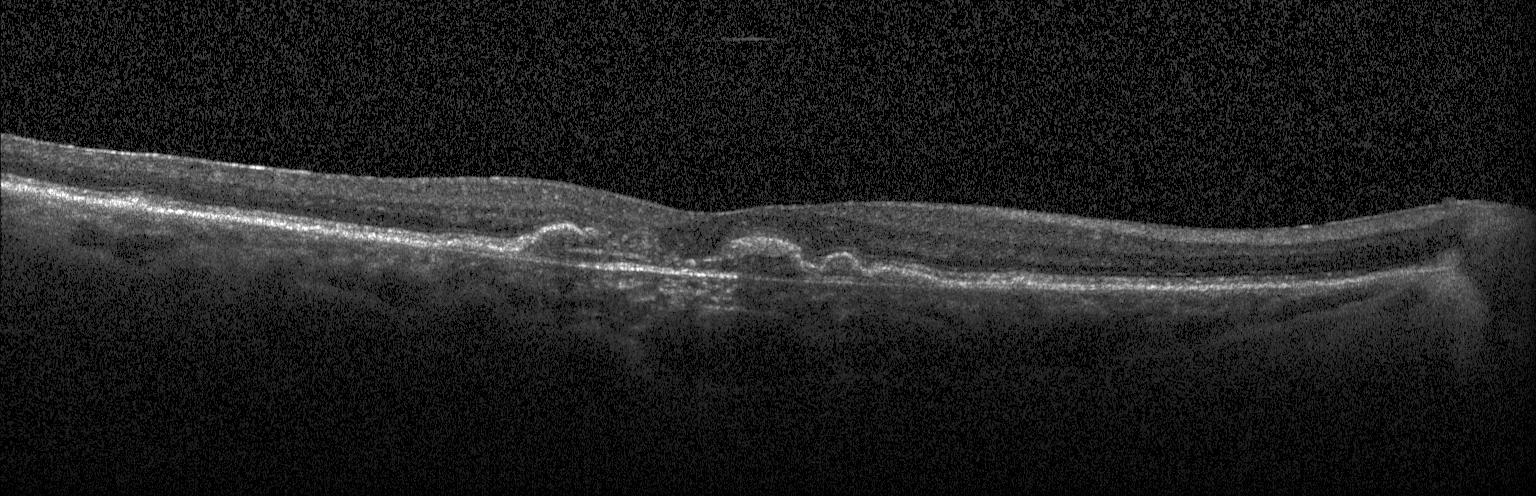 Retinal OCT cross-section, macular scan.
Diagnosis: CNV.